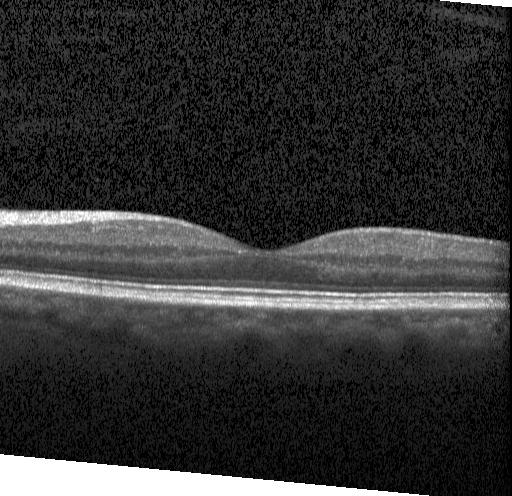

Centered on the fovea, optical coherence tomography scan, Heidelberg Spectralis. This B-scan demonstrates no choroidal neovascularization, diabetic macular edema, or drusen.